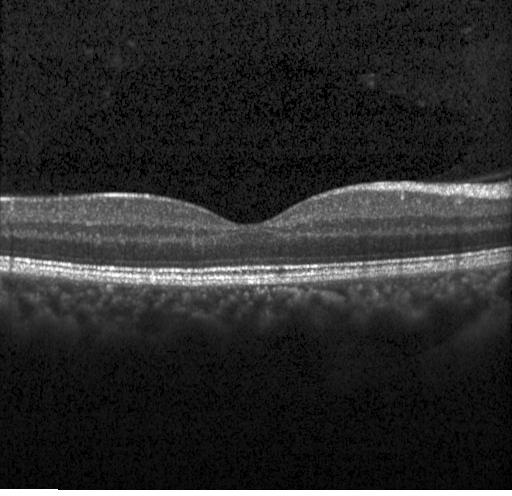
Retinal OCT B-scan, horizontal scan through the fovea, acquired on a Heidelberg Spectralis.
The scan shows no CNV, DME, or drusen.